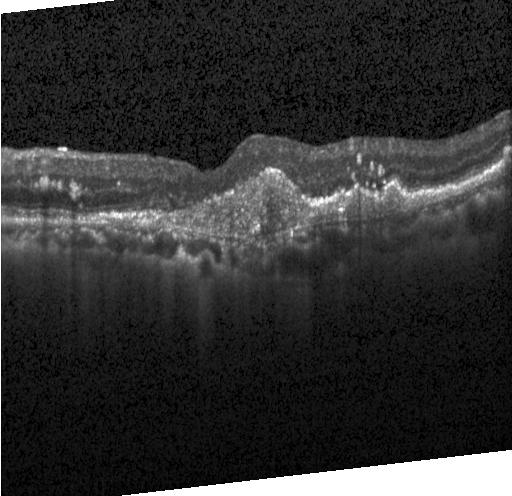 OCT finding: a choroidal neovascular membrane.